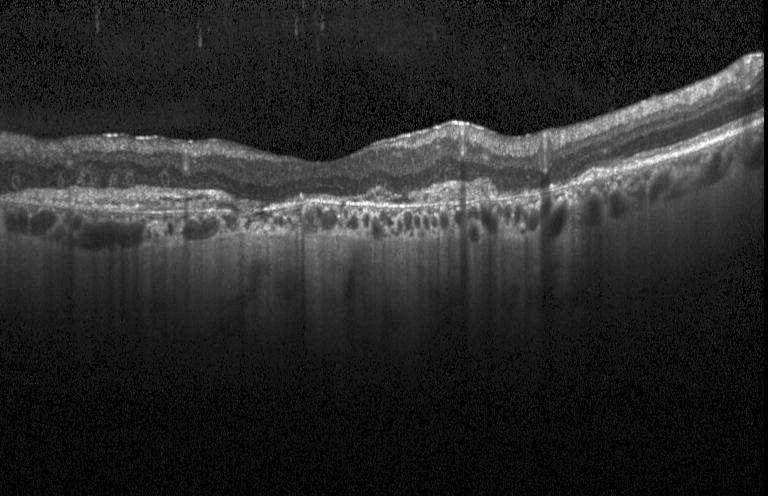 Impression: CNV.